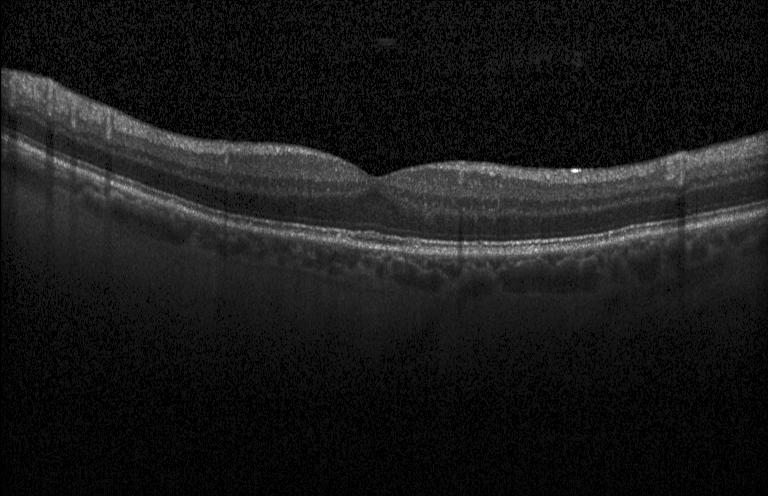
Retinal OCT cross-section.
OCT finding: no choroidal neovascularization, no diabetic macular edema, and no drusen.